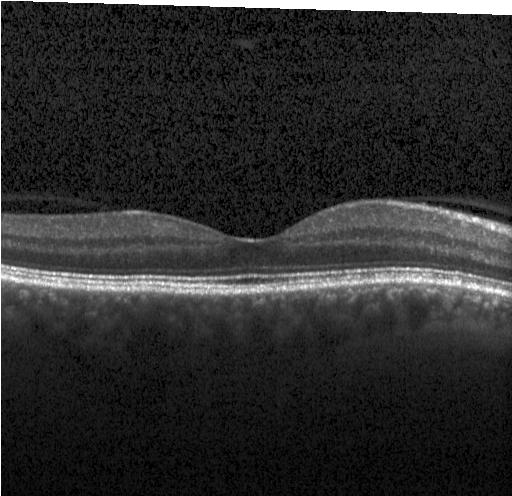 Optical coherence tomography B-scan; spectral-domain OCT. OCT finding: no CNV, DME, or drusen.